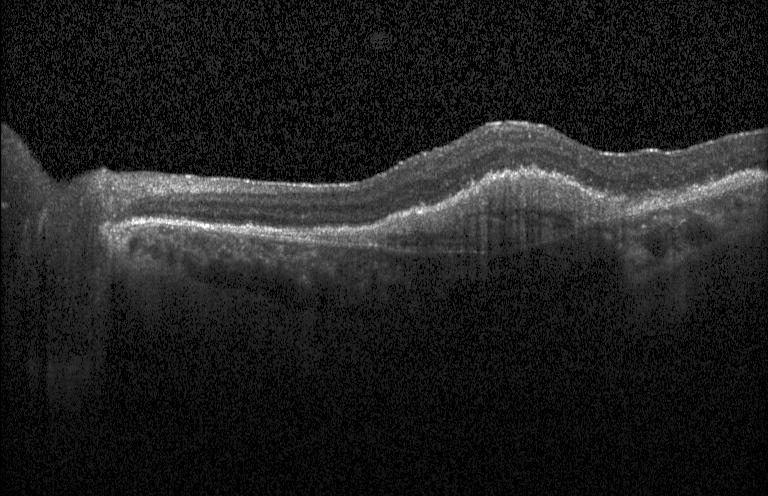

Fovea-centered; SD-OCT; instrument: Heidelberg Spectralis; optical coherence tomography scan — Finding: a choroidal neovascular membrane.